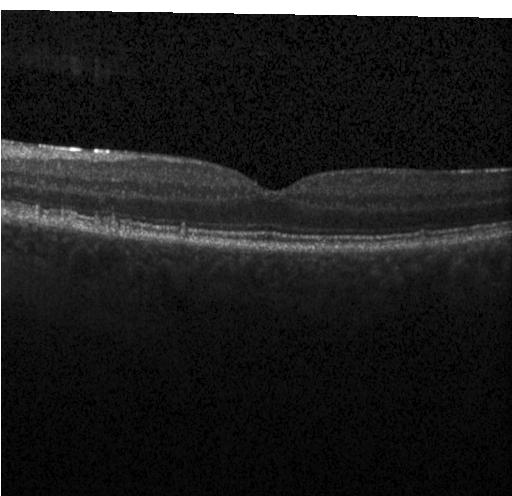 Through the macula, spectral-domain optical coherence tomography, Heidelberg Spectralis OCT system, optical coherence tomography B-scan.
This B-scan demonstrates multiple drusen.